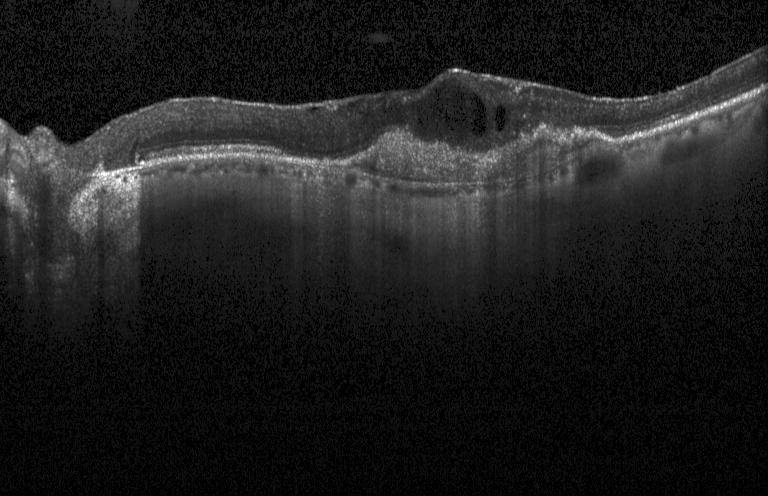
Impression: a choroidal neovascular membrane.